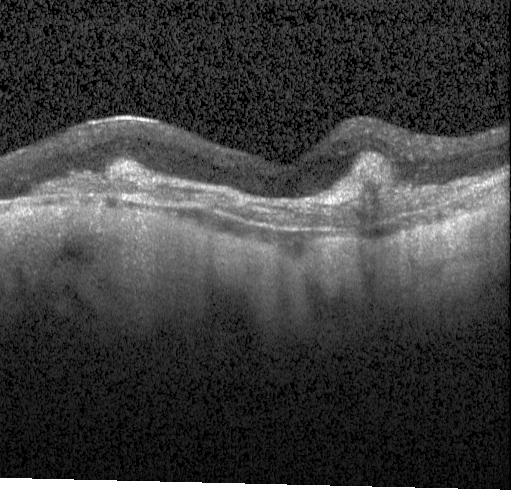
OCT finding: a choroidal neovascular membrane.